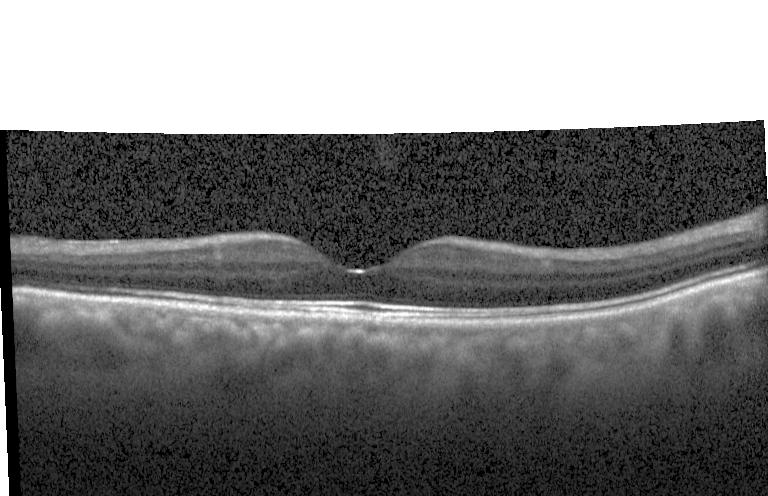

Macular scan. Heidelberg Spectralis. Spectral-domain optical coherence tomography. Optical coherence tomography scan — Neither choroidal neovascularization, diabetic macular edema, nor drusen.